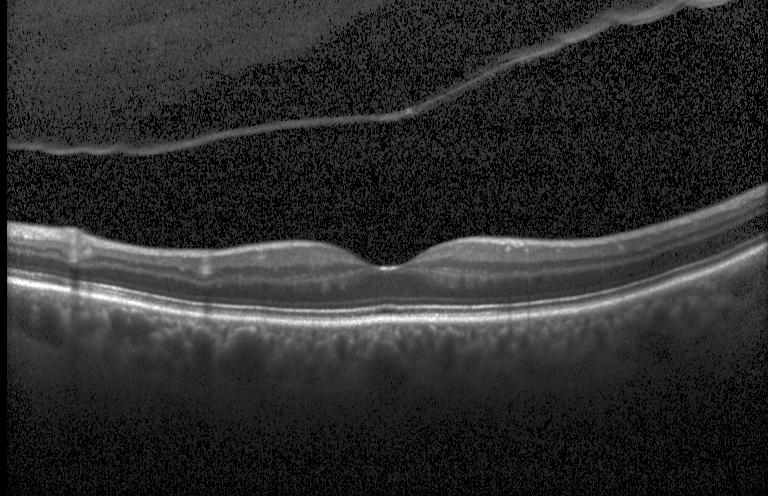
Optical coherence tomography scan. SD-OCT. Dx: no evidence of choroidal neovascularization, diabetic macular edema, or drusen.